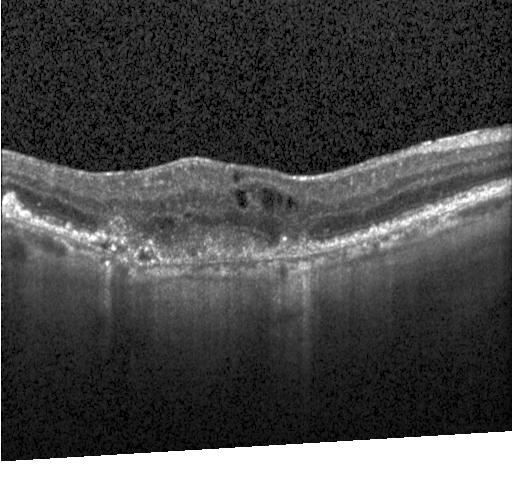 Diagnosis: CNV.